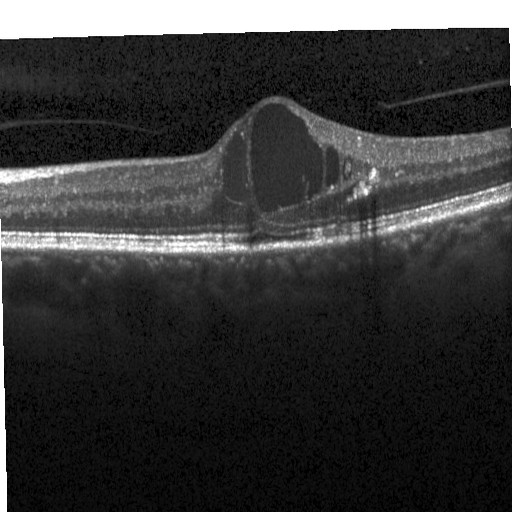

Finding: diabetic macular edema (DME).